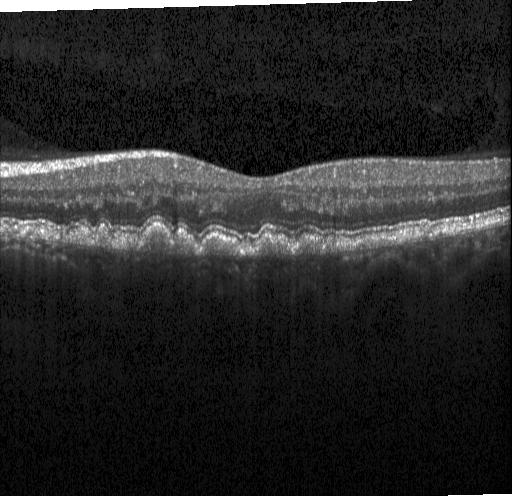
Spectral-domain OCT; retinal OCT B-scan; horizontal scan through the fovea.
This B-scan demonstrates drusen.